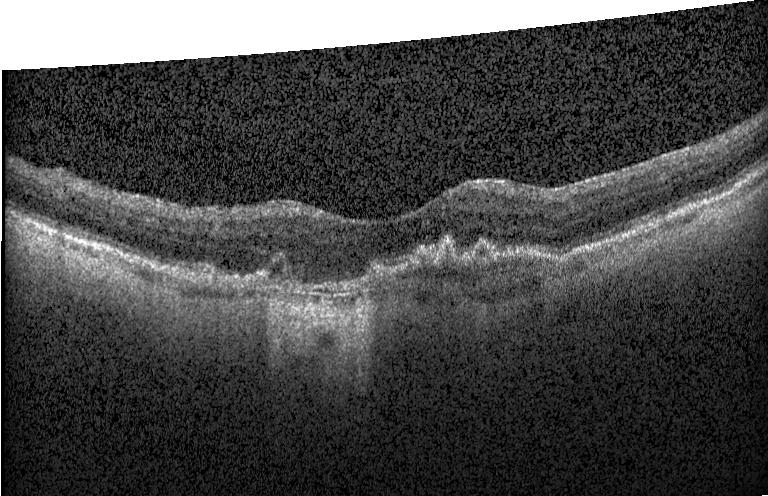
Centered on the fovea, acquired on a Heidelberg Spectralis, retinal OCT B-scan — A choroidal neovascular membrane.